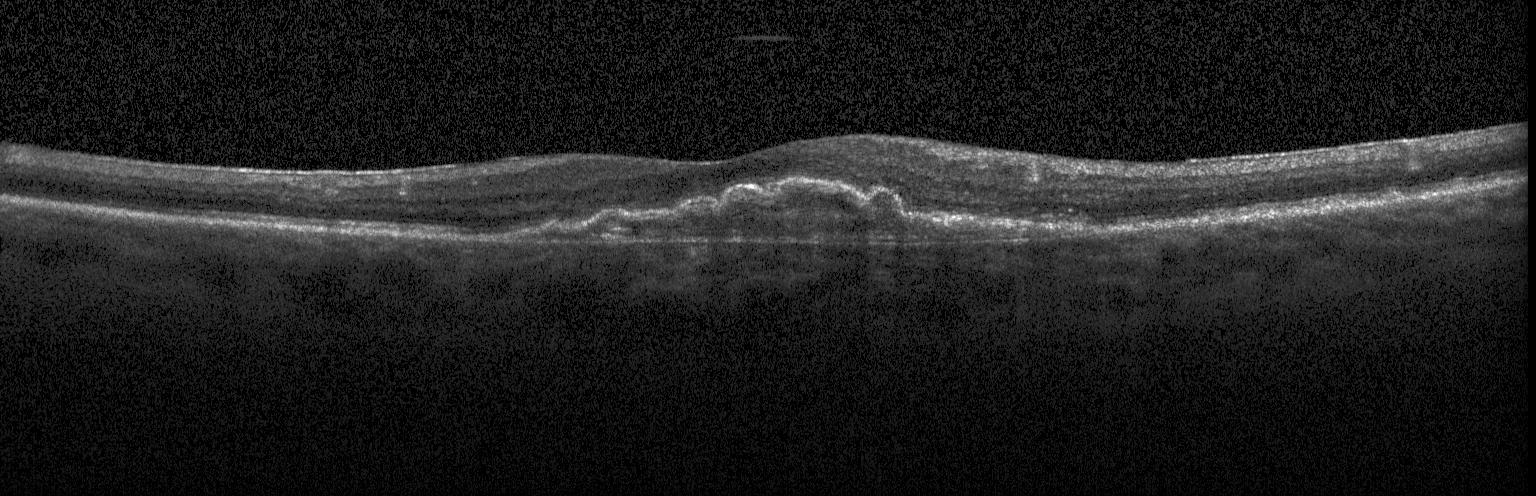
Diagnosis: choroidal neovascularization (CNV).